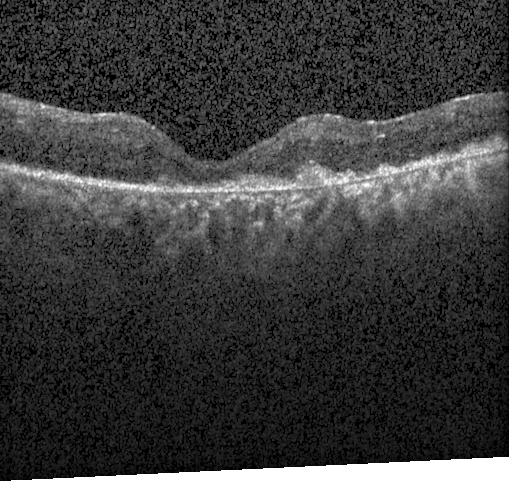

Through the macula, spectral-domain optical coherence tomography, OCT B-scan, acquired on a Heidelberg Spectralis. OCT finding: a choroidal neovascular membrane.